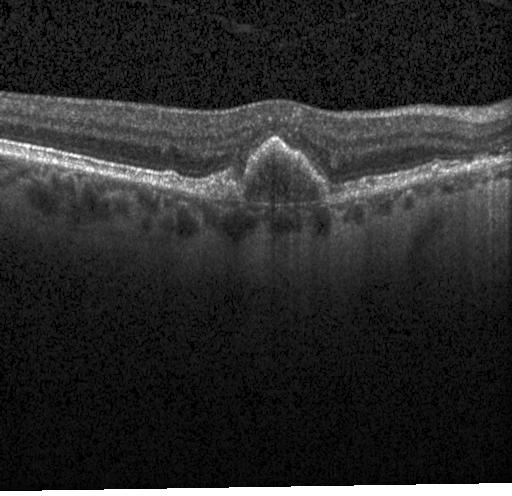 OCT line scan; SD-OCT; Heidelberg Spectralis.
A choroidal neovascular membrane.